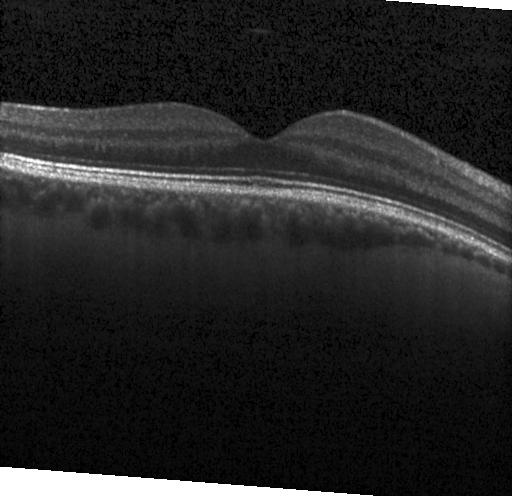 Dx: no CNV, no DME, and no drusen.